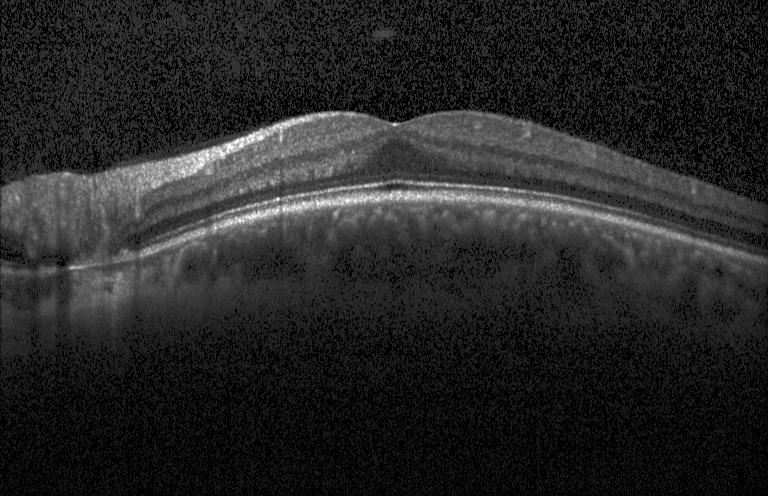
Spectral-domain OCT. Centered on the fovea. Retinal OCT B-scan.
Impression: no evidence of choroidal neovascularization, diabetic macular edema, or drusen.